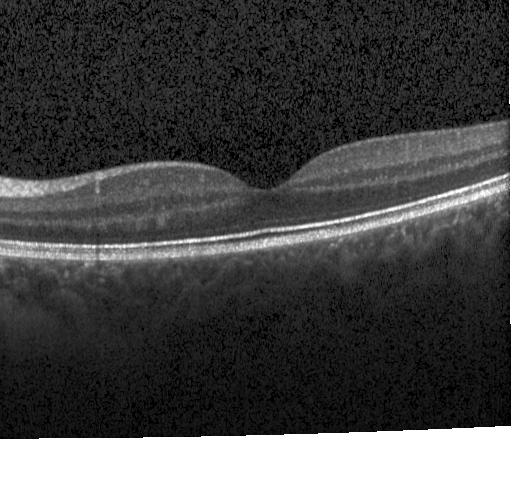 OCT B-scan; horizontal scan through the fovea. This B-scan demonstrates neither choroidal neovascularization, diabetic macular edema, nor drusen.